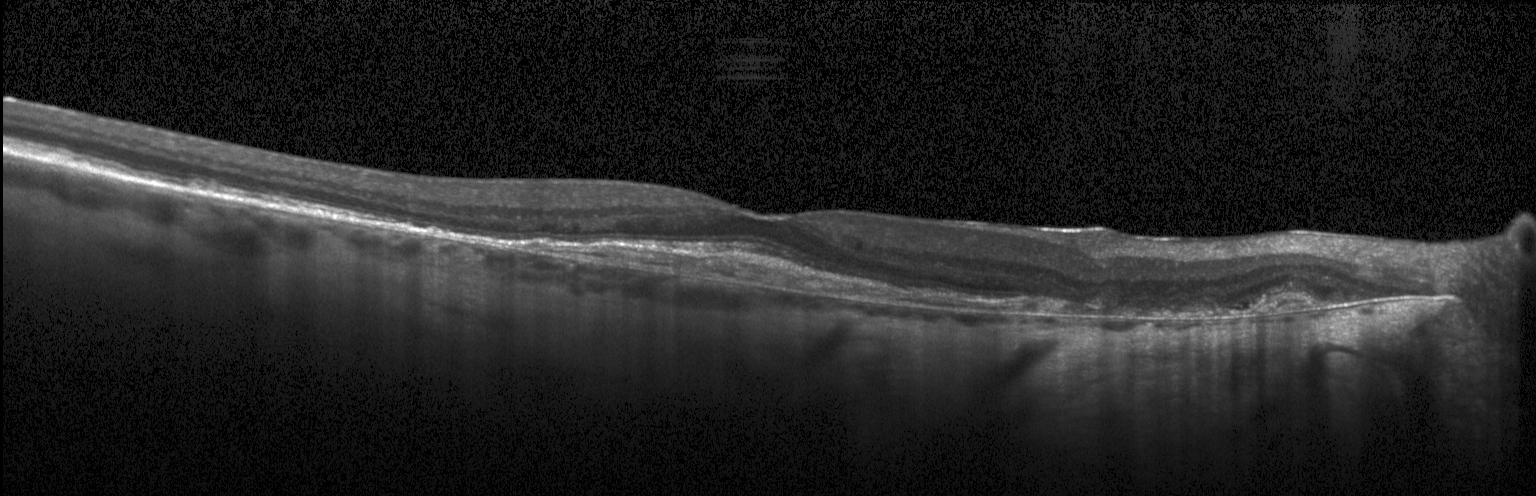
Spectral-domain OCT, optical coherence tomography scan, Heidelberg Spectralis
OCT finding: a choroidal neovascular membrane.